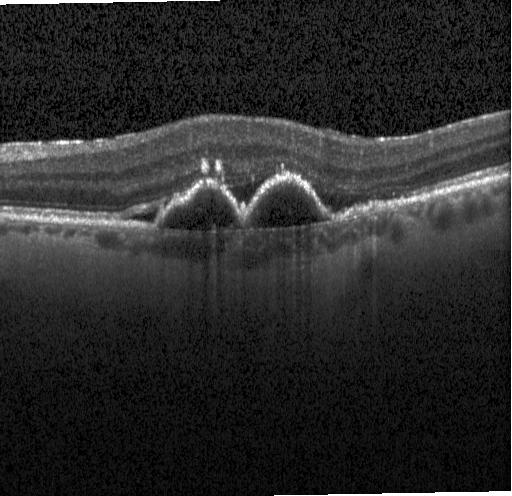
Centered on the fovea, OCT line scan, SD-OCT, acquired on a Heidelberg Spectralis.
Diagnosis: a choroidal neovascular membrane.